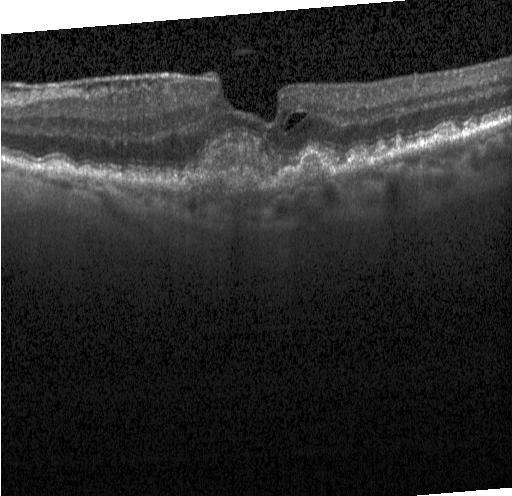

Spectral-domain OCT. Retinal OCT B-scan
This B-scan demonstrates a choroidal neovascular membrane.